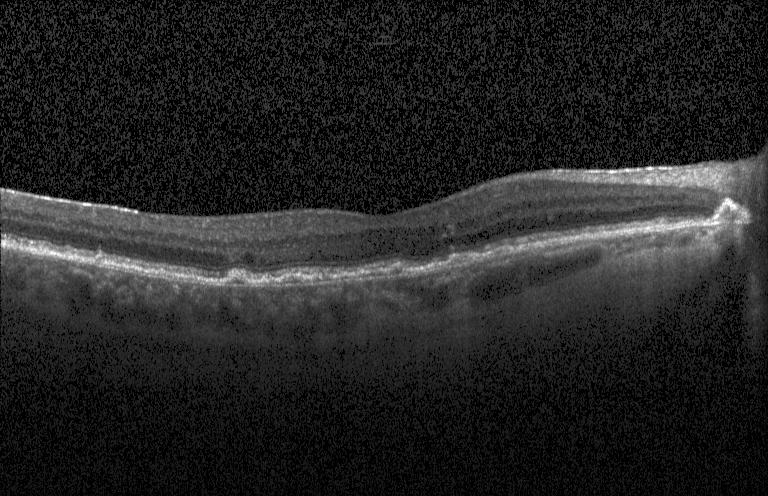 Macular OCT: a choroidal neovascular membrane.